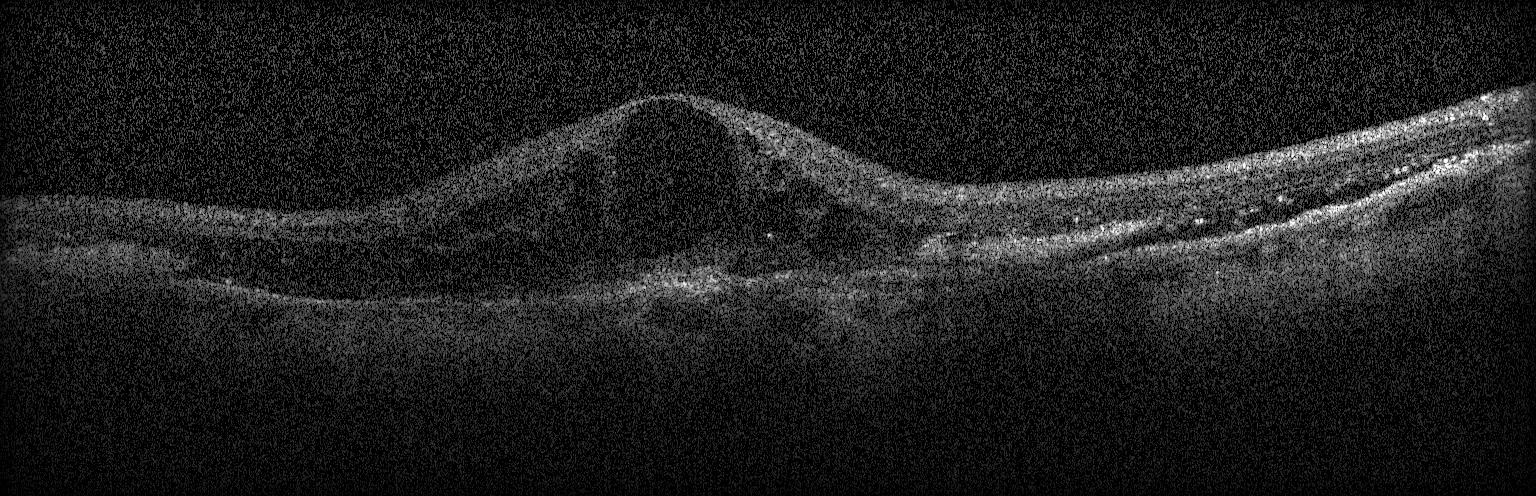
Macular OCT: a choroidal neovascular membrane.